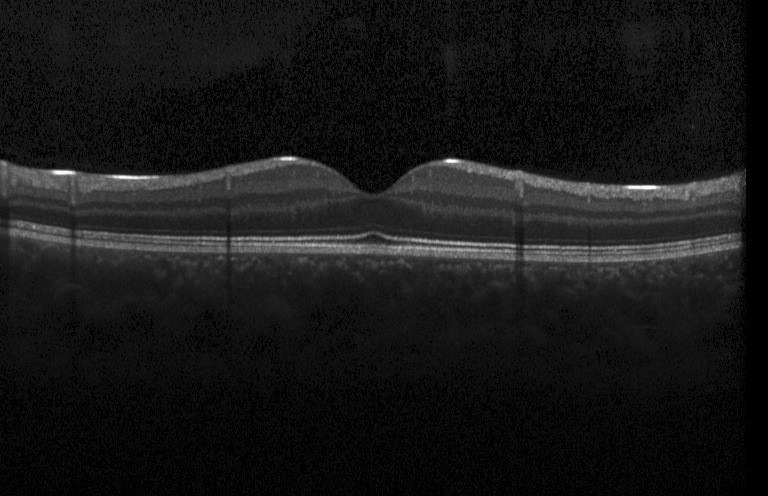 OCT scan showing neither CNV, DME, nor drusen.